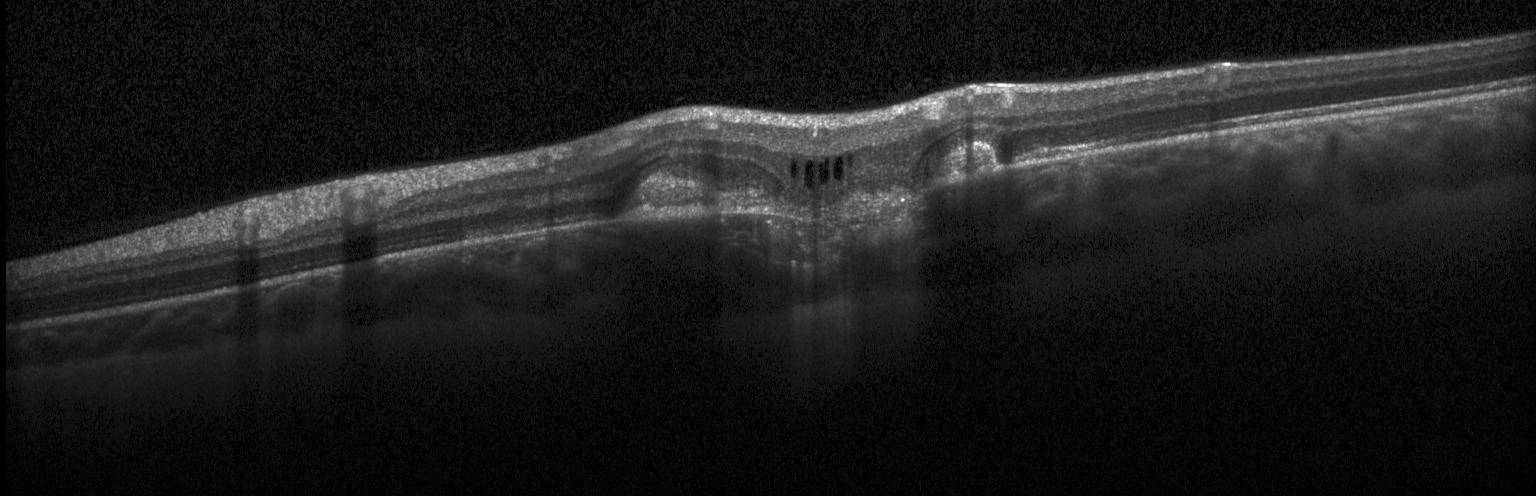
Diagnosis: choroidal neovascularization (CNV).